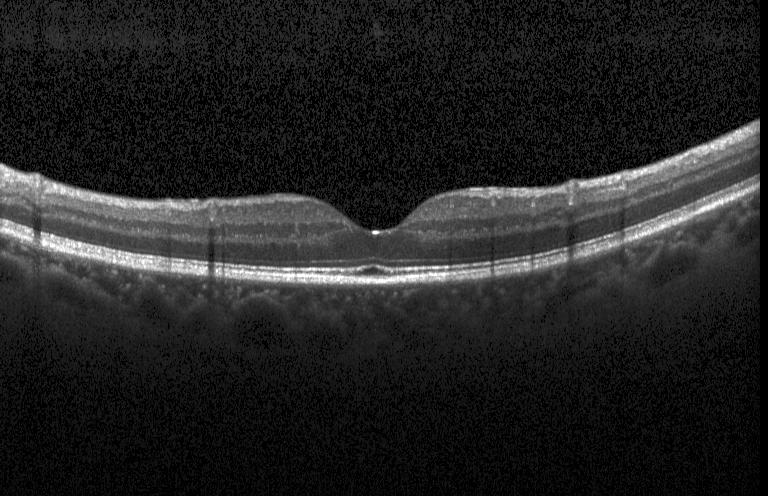 Impression: no choroidal neovascularization, no diabetic macular edema, and no drusen.